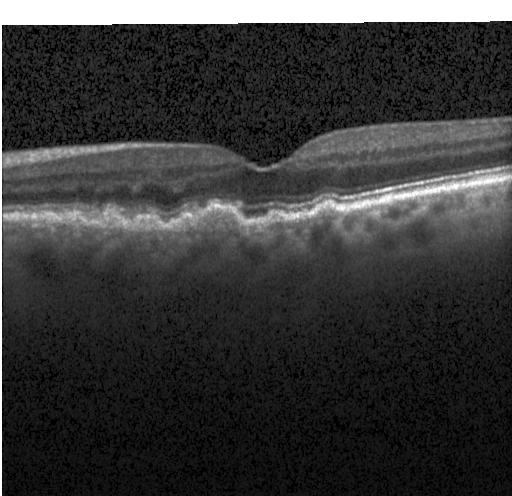 Optical coherence tomography B-scan — Macular OCT: multiple drusen.